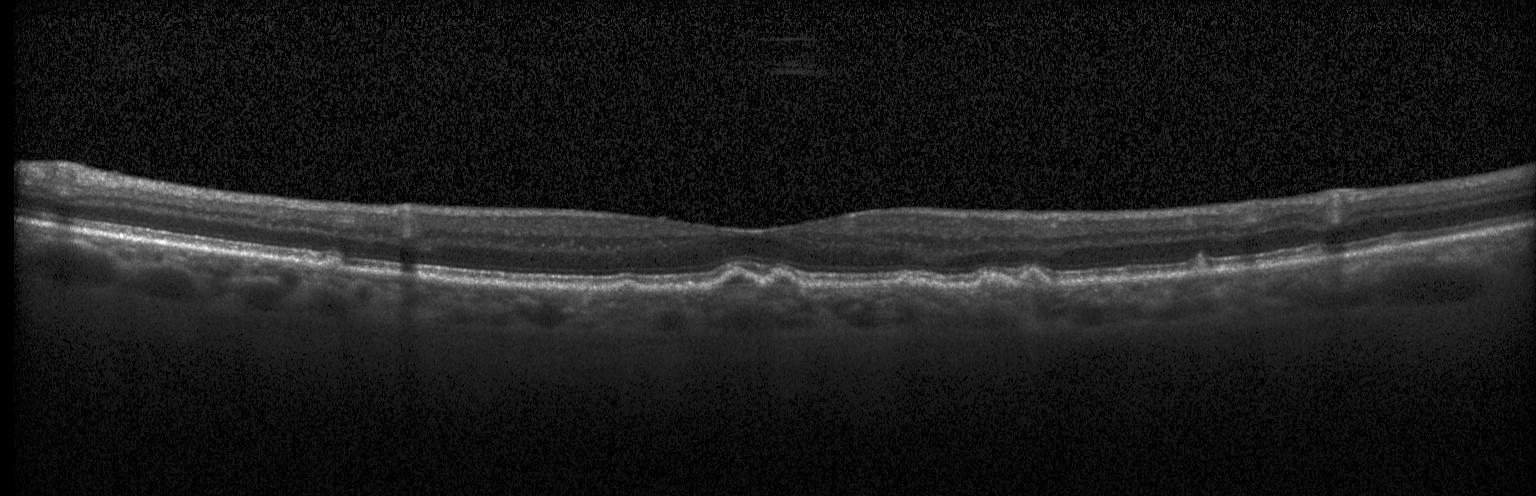 Dx: choroidal neovascularization (CNV).